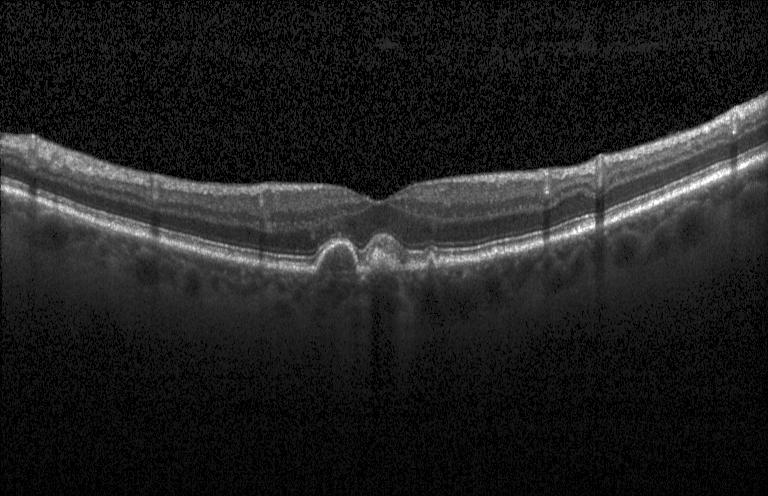
OCT finding: choroidal neovascularization (CNV).